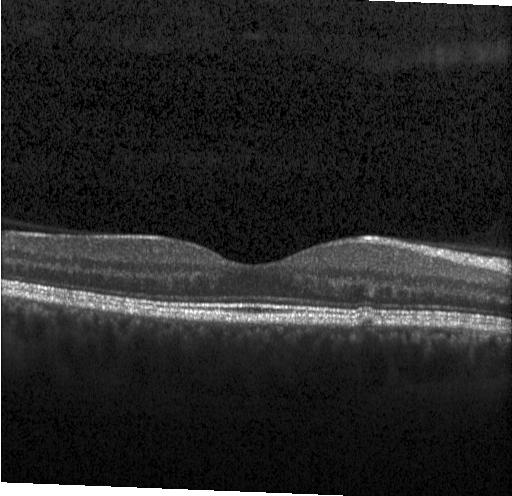
Optical coherence tomography scan. Fovea-centered — Impression: multiple drusen.